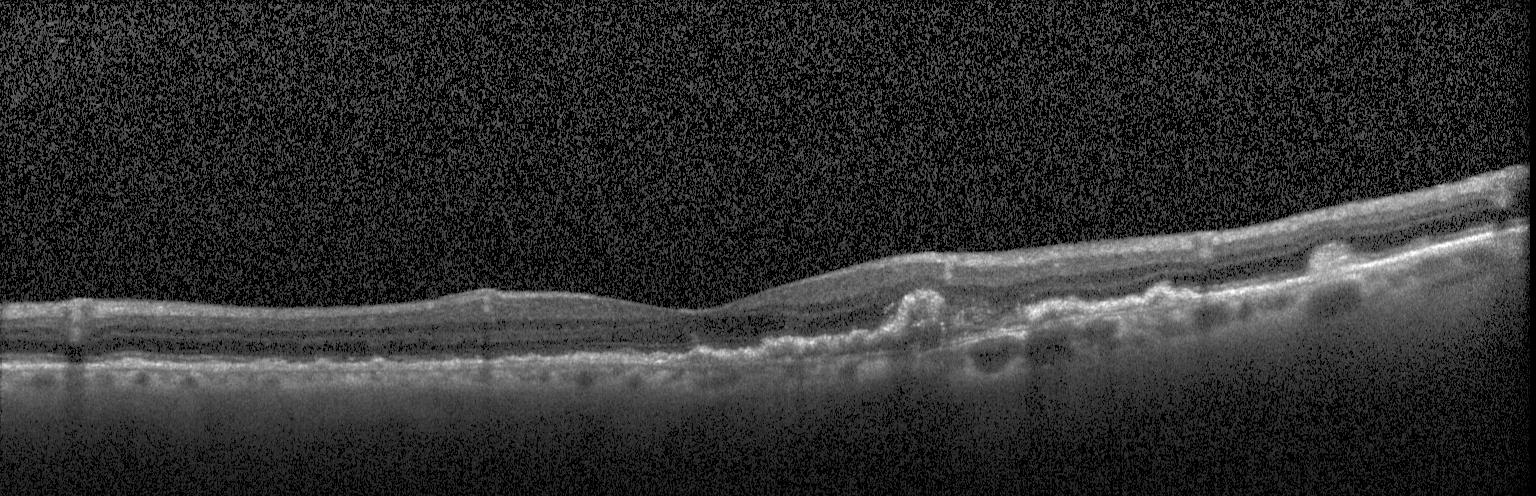
Retinal OCT cross-section showing CNV.